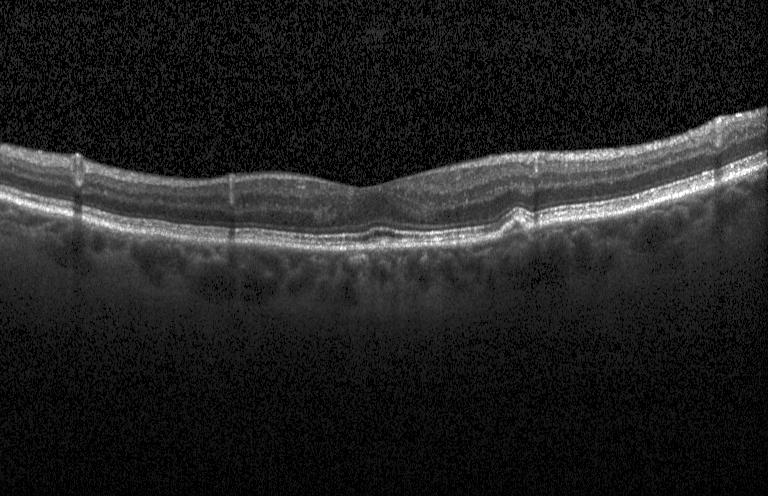
Centered on the fovea, OCT B-scan, acquired on a Heidelberg Spectralis. Dx: multiple drusen.